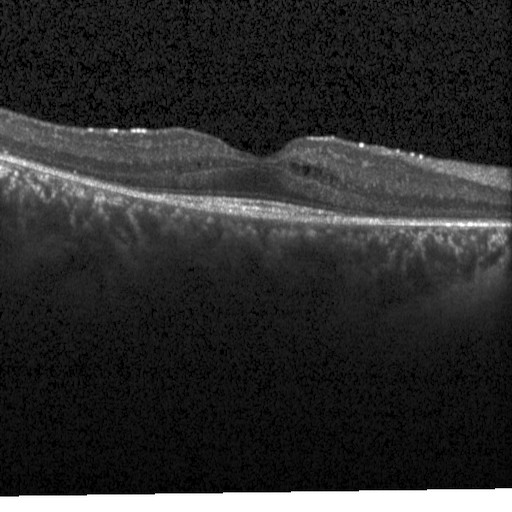 Impression: diabetic macular edema (DME).